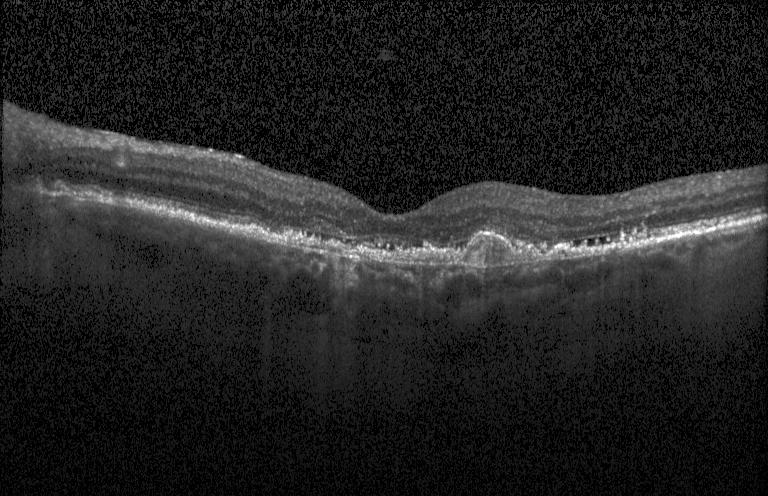
OCT line scan · acquired on a Heidelberg Spectralis · spectral-domain optical coherence tomography · centered on the fovea. OCT finding: a choroidal neovascular membrane.